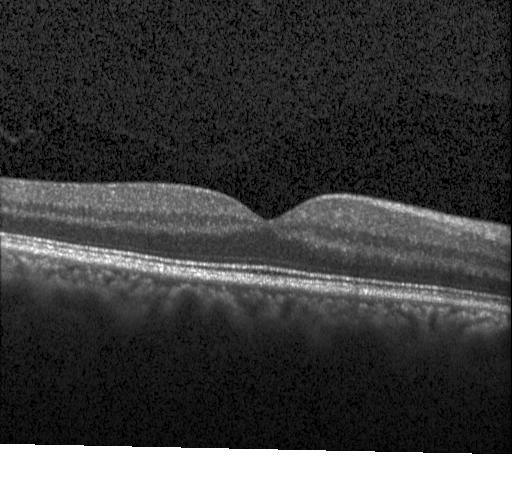 Instrument: Heidelberg Spectralis, OCT B-scan — Finding: no choroidal neovascularization, no diabetic macular edema, and no drusen.